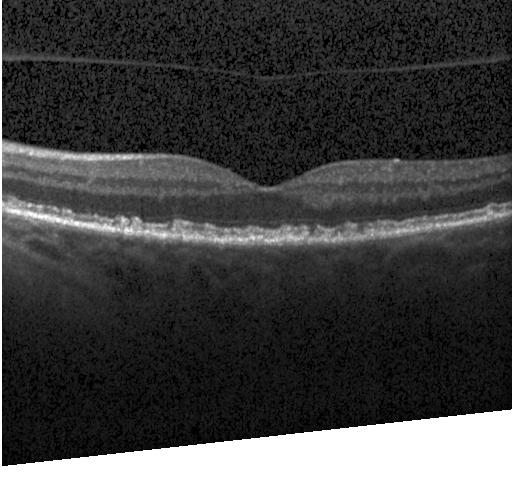
Optical coherence tomography scan, instrument: Heidelberg Spectralis, horizontal scan through the fovea, spectral-domain optical coherence tomography
Diagnosis: drusen.